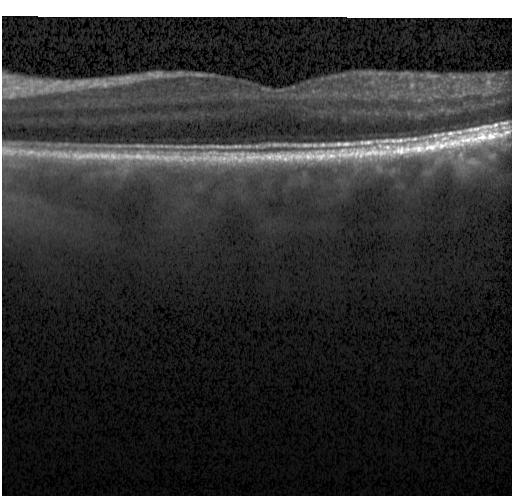

Heidelberg Spectralis OCT system. Retinal OCT cross-section. No evidence of choroidal neovascularization, diabetic macular edema, or drusen.